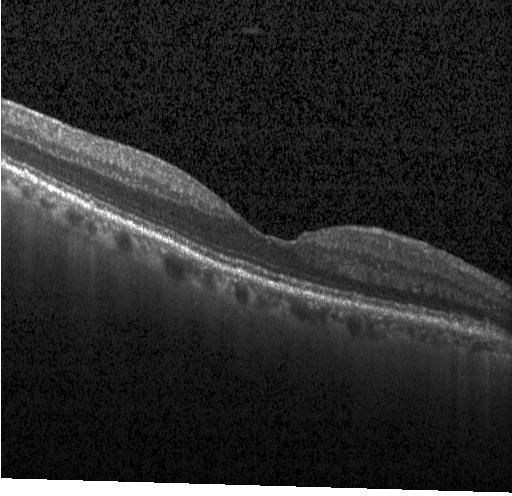 OCT line scan. Macular OCT: no evidence of CNV, DME, or drusen.